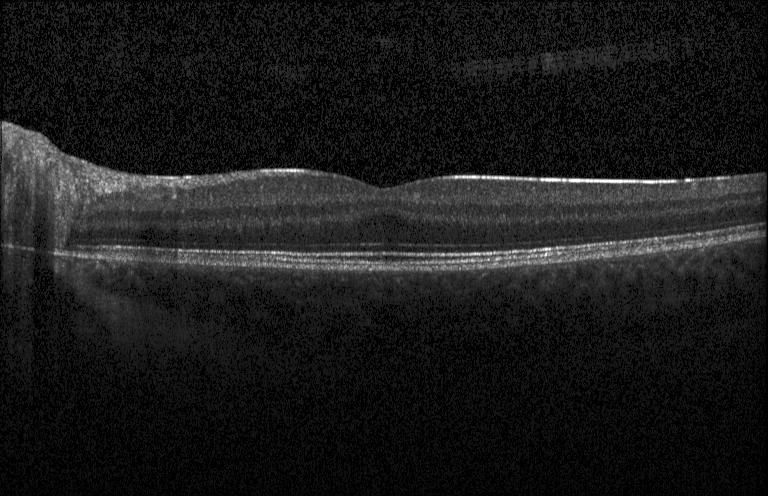

Spectral-domain OCT B-scan: no CNV, DME, or drusen.